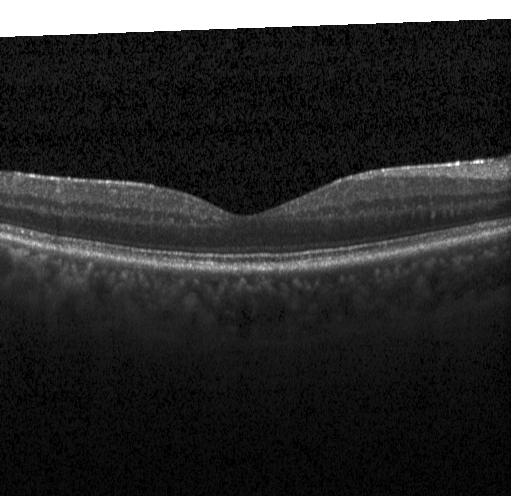 Optical coherence tomography B-scan. Spectral-domain OCT. Fovea-centered — This B-scan demonstrates no CNV, no DME, and no drusen.